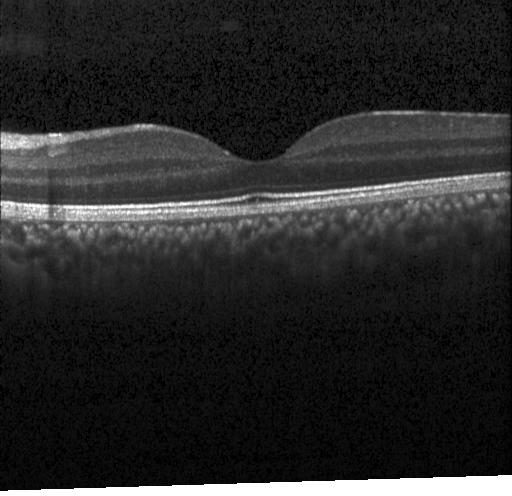

Retinal OCT cross-section — Assessment: neither CNV, DME, nor drusen.